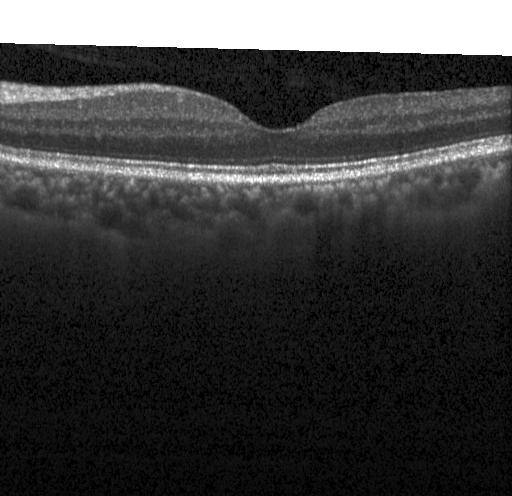
OCT line scan; horizontal scan through the fovea; acquired on a Heidelberg Spectralis.
Assessment: no evidence of choroidal neovascularization, diabetic macular edema, or drusen.